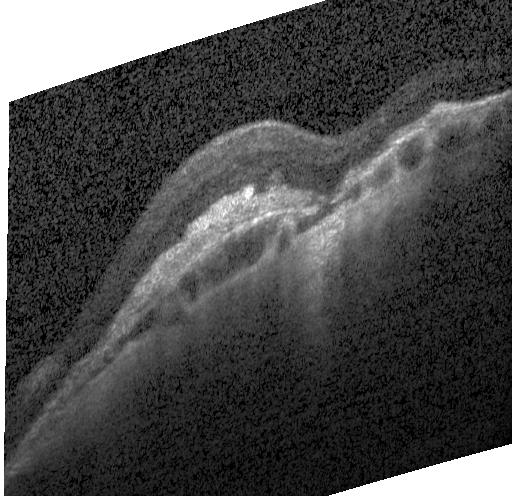

Assessment: a choroidal neovascular membrane.